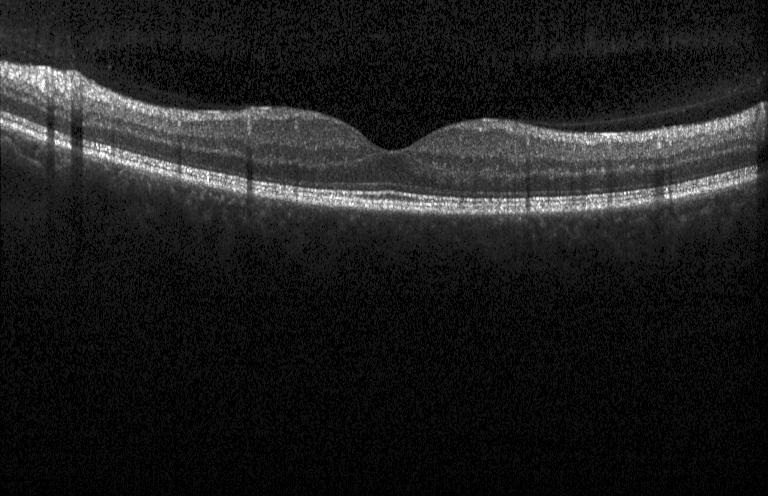

OCT line scan.
Impression: no evidence of choroidal neovascularization, diabetic macular edema, or drusen.